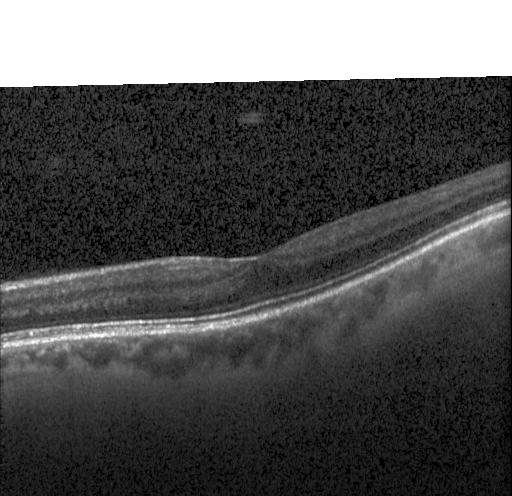 OCT line scan.
The scan shows no choroidal neovascularization, diabetic macular edema, or drusen.